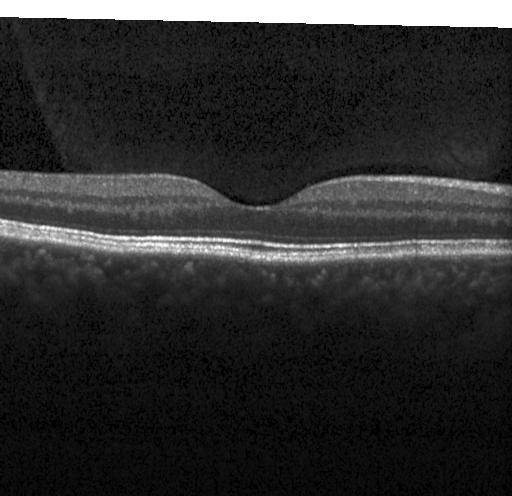
Retinal OCT cross-section showing no choroidal neovascularization, no diabetic macular edema, and no drusen.